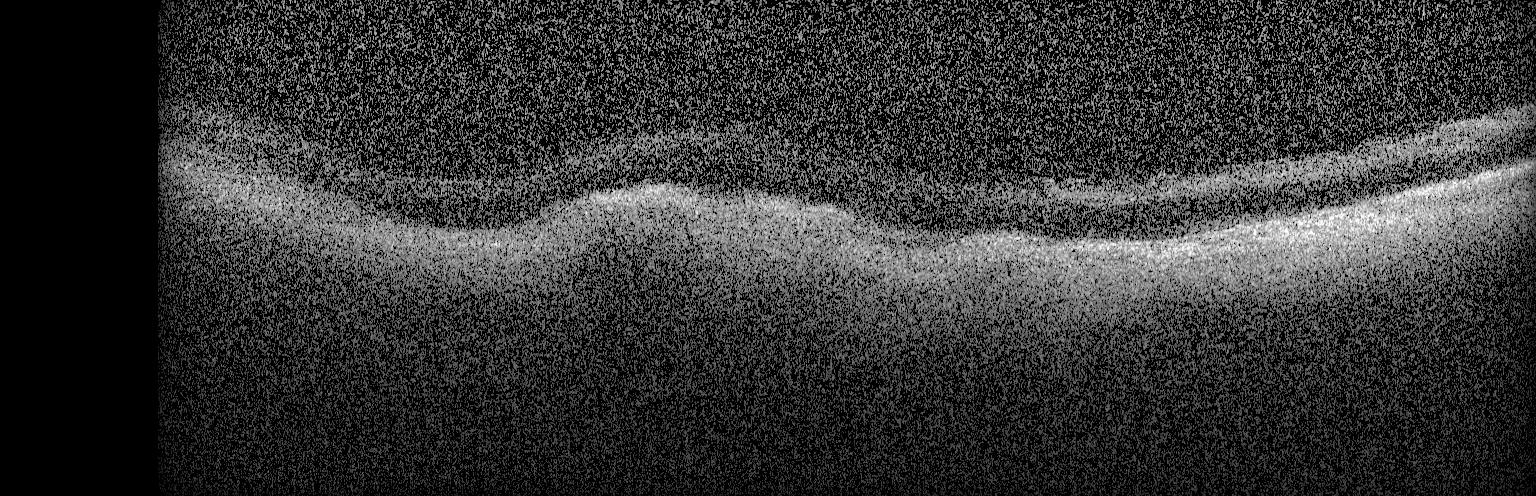

SD-OCT; OCT B-scan; instrument: Heidelberg Spectralis.
Finding: choroidal neovascularization.